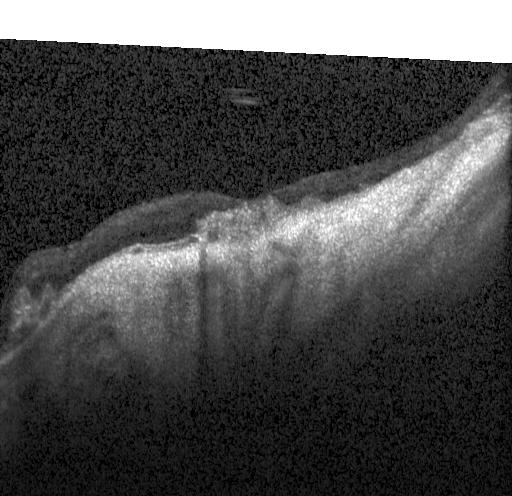
The scan shows a choroidal neovascular membrane.